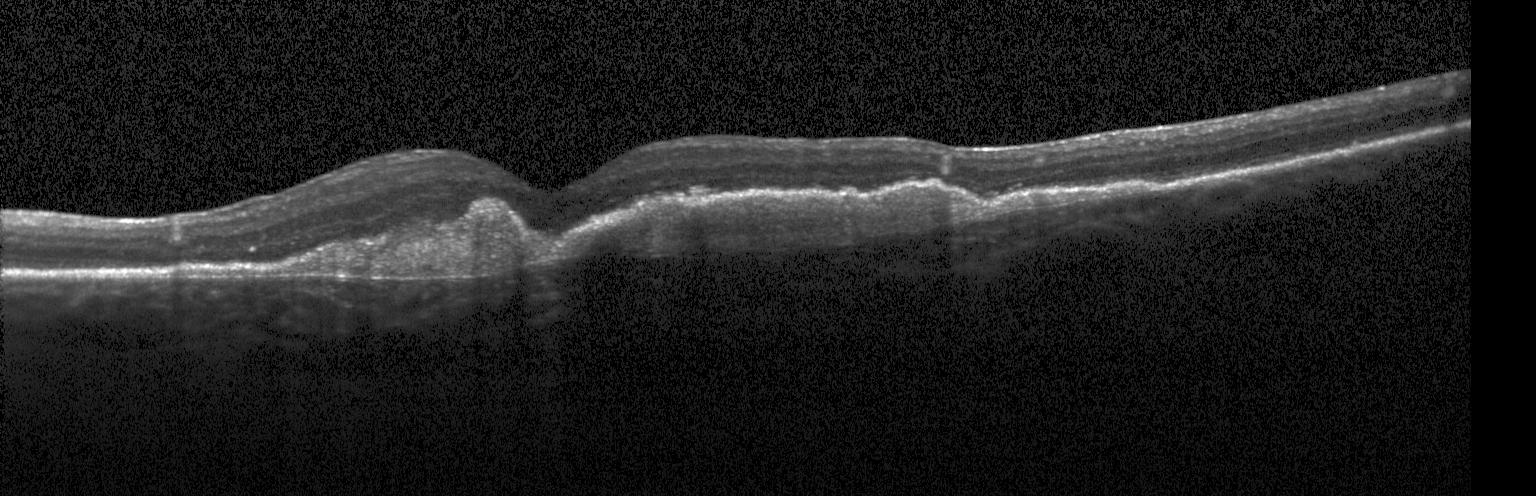

OCT line scan, through the macula.
Finding: choroidal neovascularization (CNV).